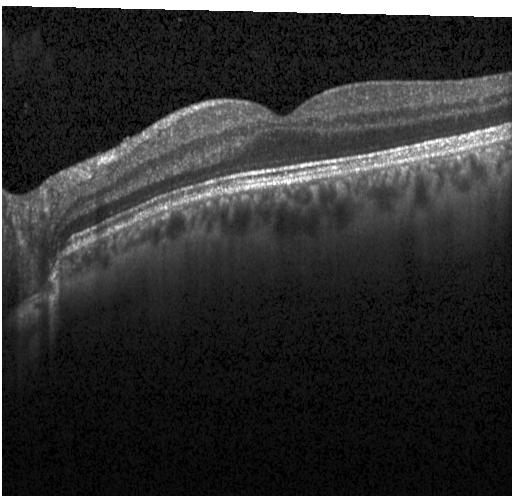

OCT line scan — Impression: no choroidal neovascularization, no diabetic macular edema, and no drusen.